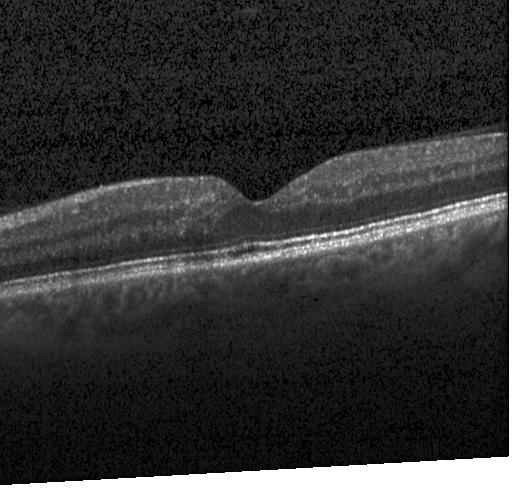

OCT B-scan. Macular OCT: no CNV, no DME, and no drusen.